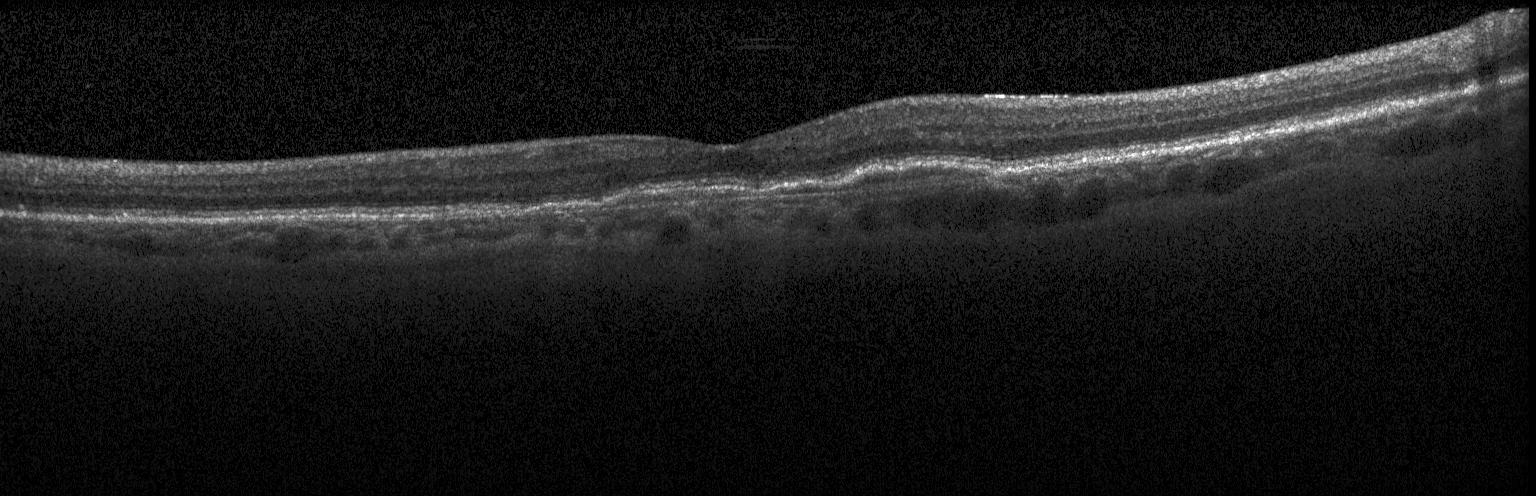

SD-OCT; OCT line scan
Assessment: CNV.